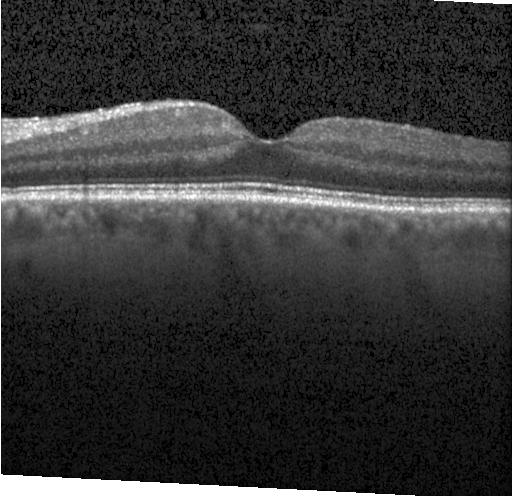

OCT B-scan, spectral-domain optical coherence tomography — Impression: no evidence of choroidal neovascularization, diabetic macular edema, or drusen.